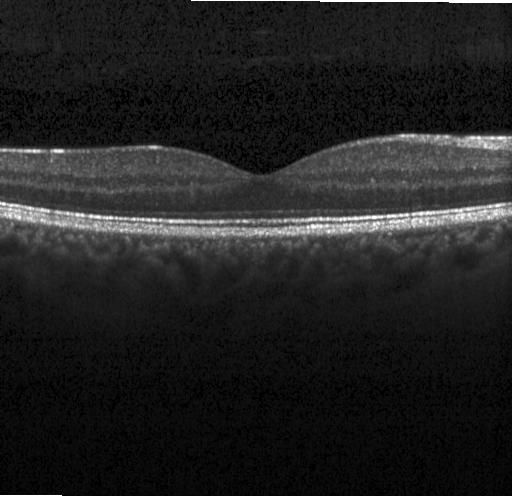
Assessment: no choroidal neovascularization, diabetic macular edema, or drusen.